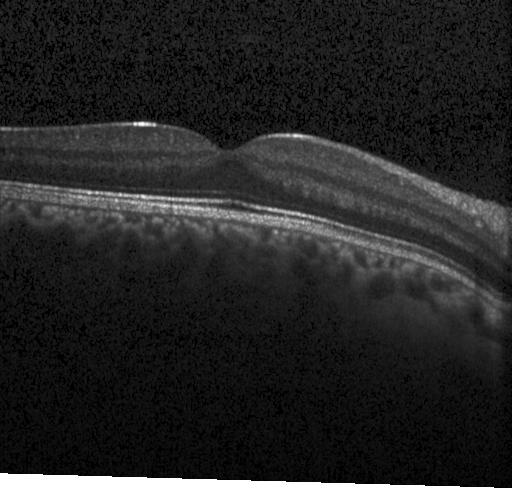
Optical coherence tomography scan, centered on the fovea, SD-OCT.
Macular OCT: no evidence of choroidal neovascularization, diabetic macular edema, or drusen.